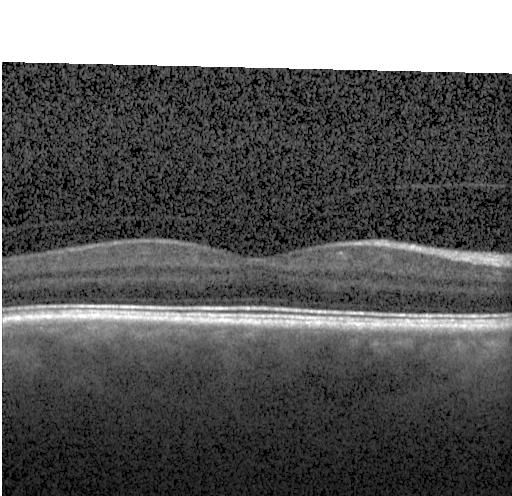
Finding: no choroidal neovascularization, diabetic macular edema, or drusen.